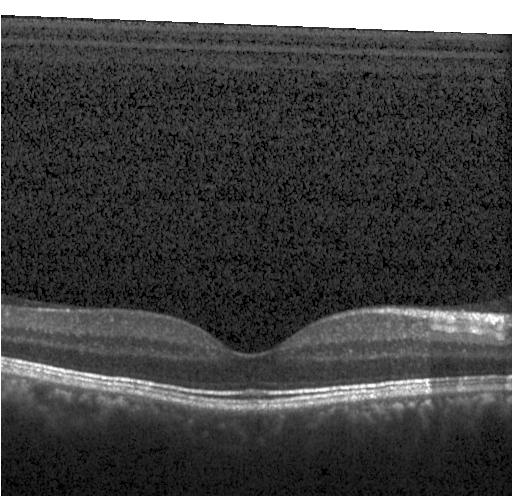

Retinal OCT B-scan
No choroidal neovascularization, diabetic macular edema, or drusen.